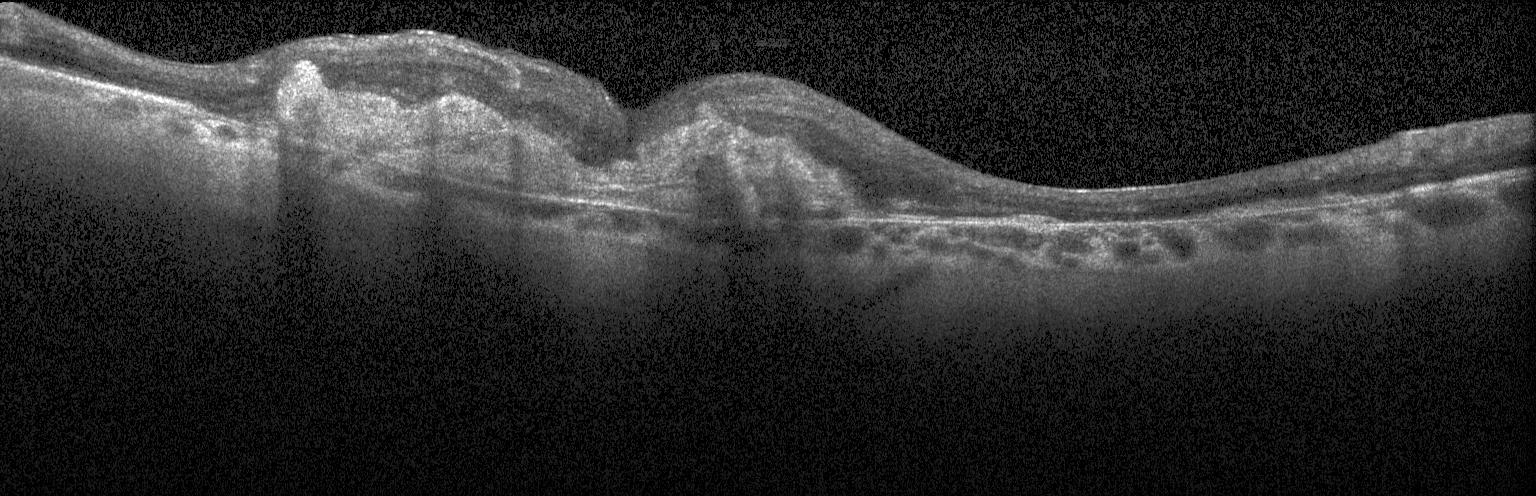
Impression: CNV.